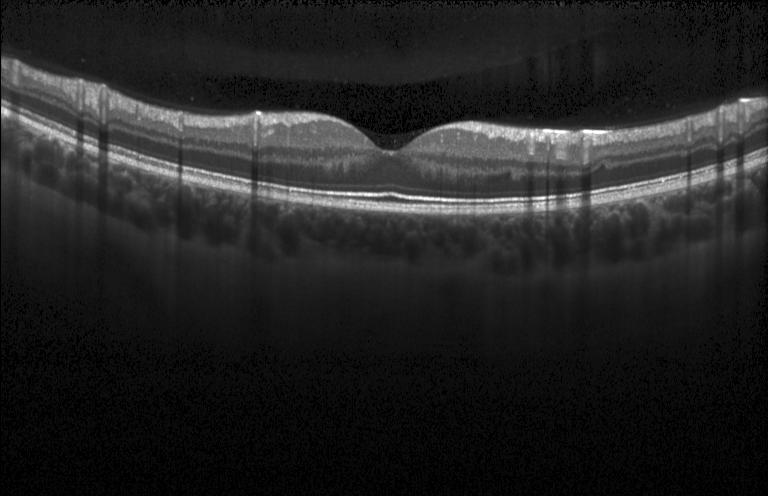 OCT B-scan showing no evidence of CNV, DME, or drusen.